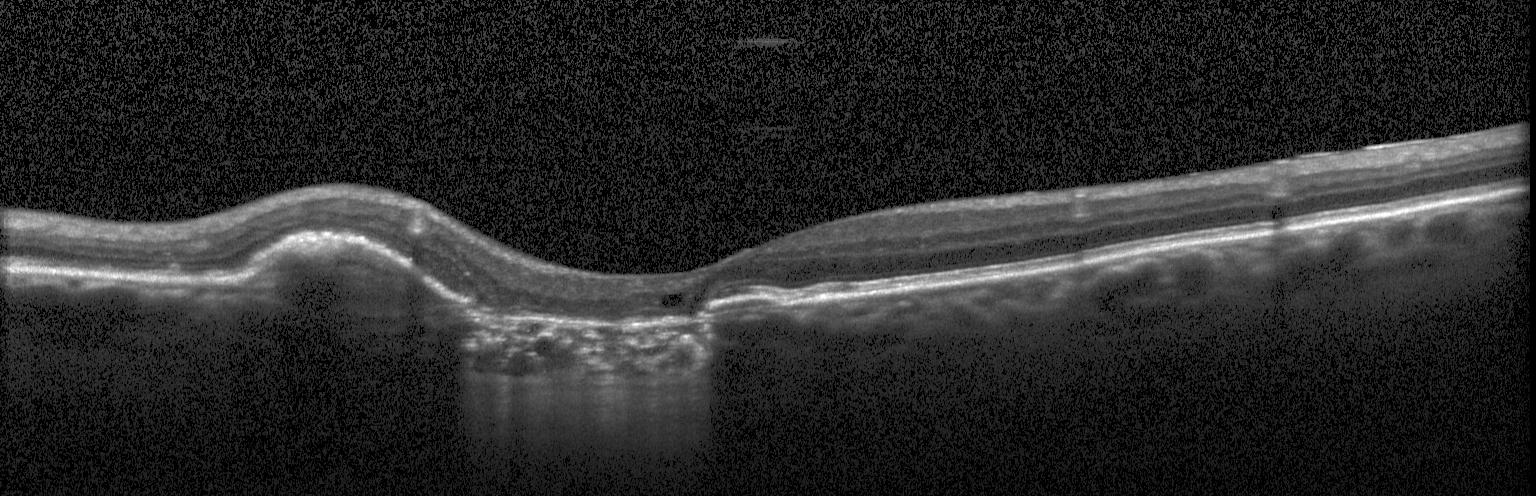 Macular OCT demonstrating a choroidal neovascular membrane.